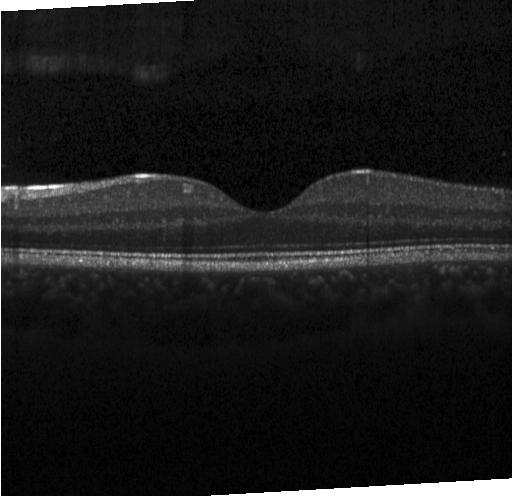
Spectral-domain OCT · optical coherence tomography B-scan. Diagnosis: no evidence of CNV, DME, or drusen.